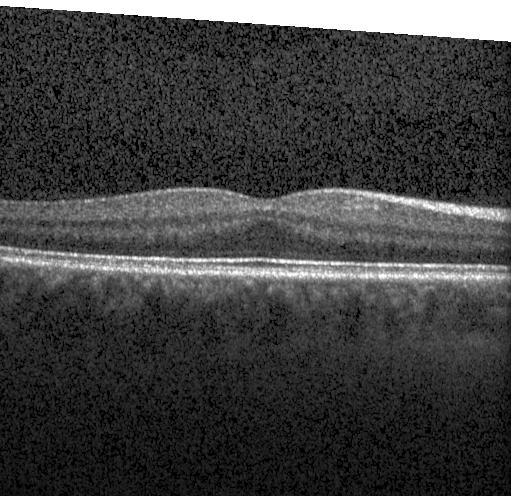
The scan shows neither CNV, DME, nor drusen.